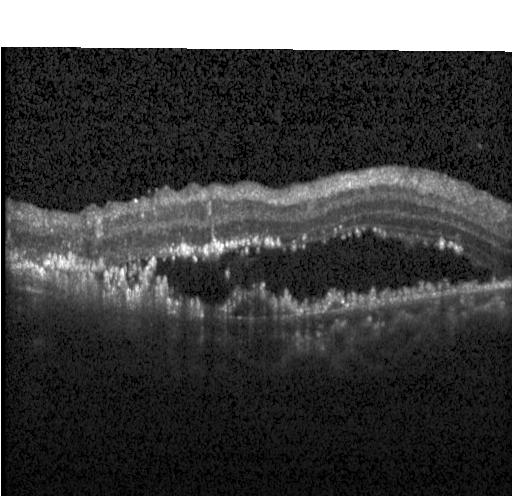
Optical coherence tomography scan, macular scan, spectral-domain optical coherence tomography.
Dx: a choroidal neovascular membrane.